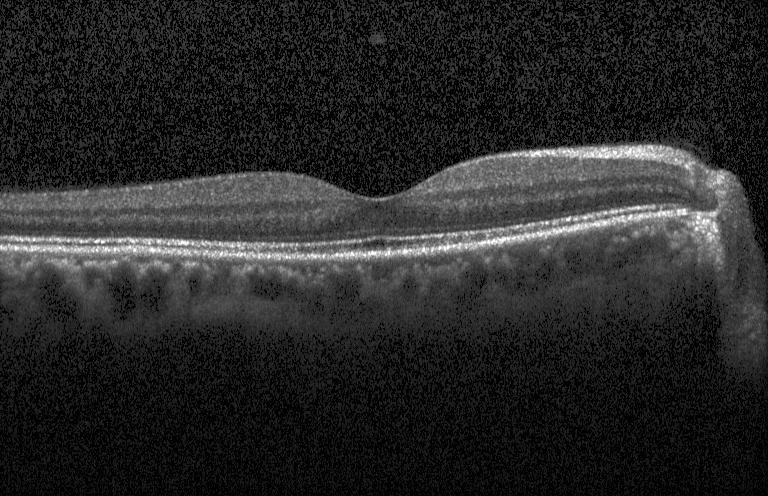

Retinal OCT B-scan. Heidelberg Spectralis
This B-scan demonstrates no CNV, DME, or drusen.